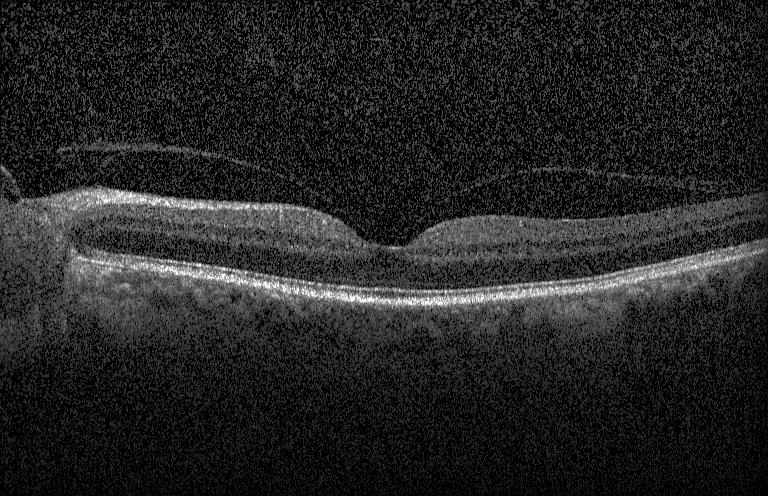

OCT B-scan showing no evidence of choroidal neovascularization, diabetic macular edema, or drusen.